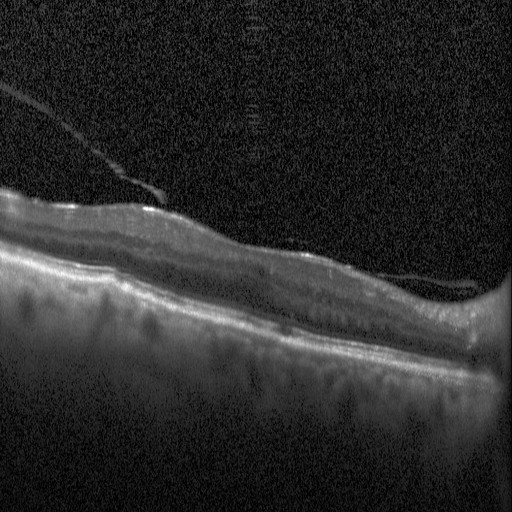
Heidelberg Spectralis · optical coherence tomography B-scan · spectral-domain OCT · centered on the fovea — Dx: diabetic macular edema (DME).